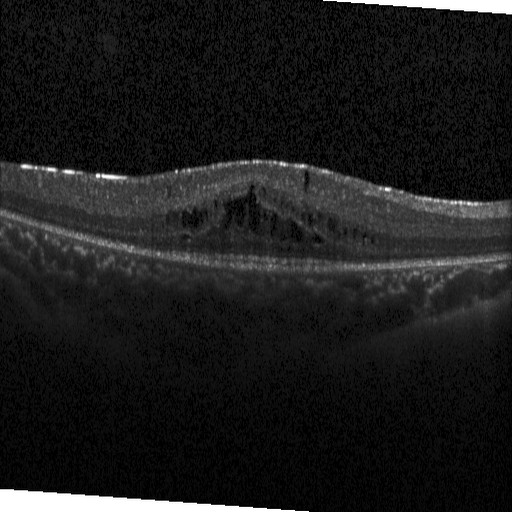 Diagnosis: diabetic macular edema.